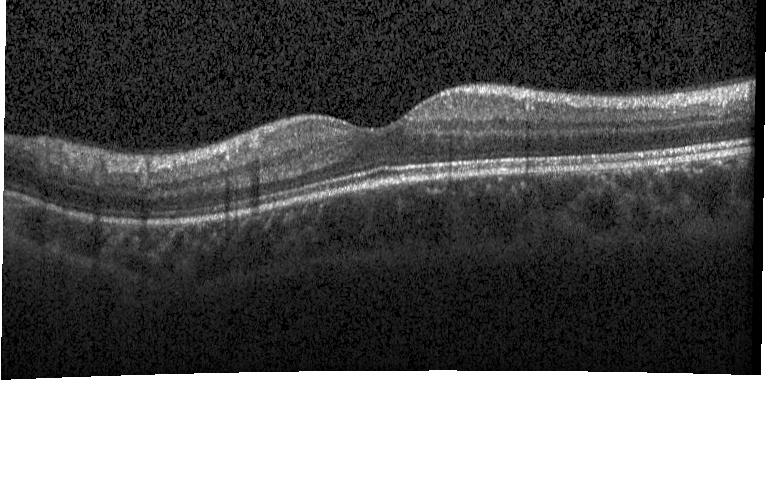

Retinal OCT cross-section — Dx: no CNV, no DME, and no drusen.